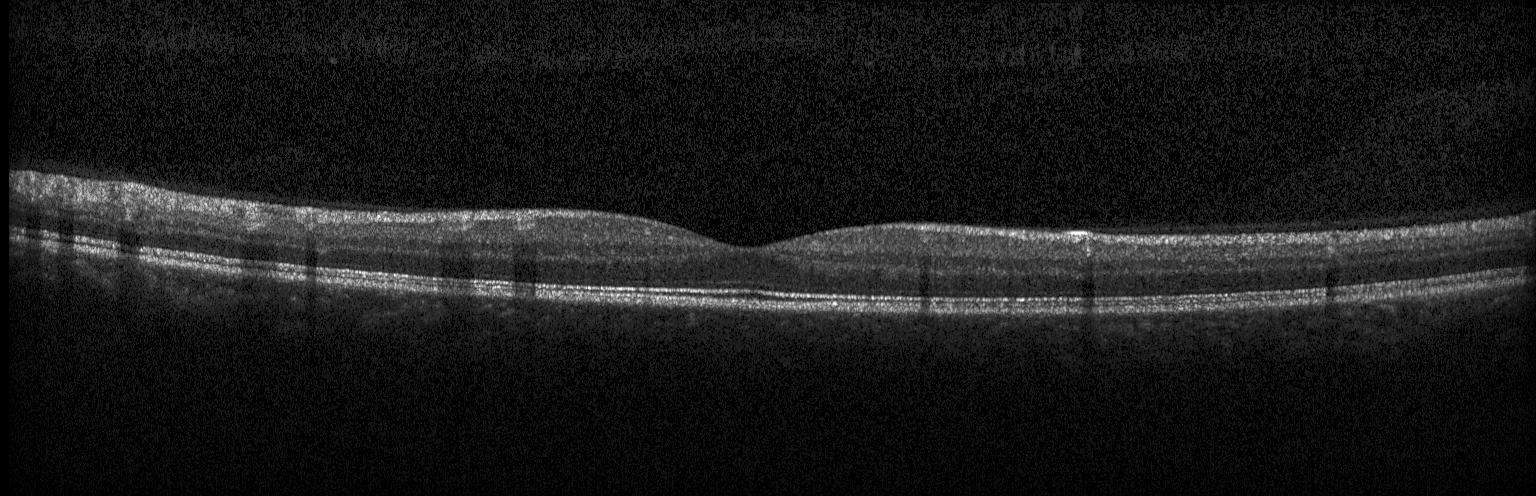

OCT B-scan. Macular scan. Heidelberg Spectralis
Diagnosis: no choroidal neovascularization, diabetic macular edema, or drusen.